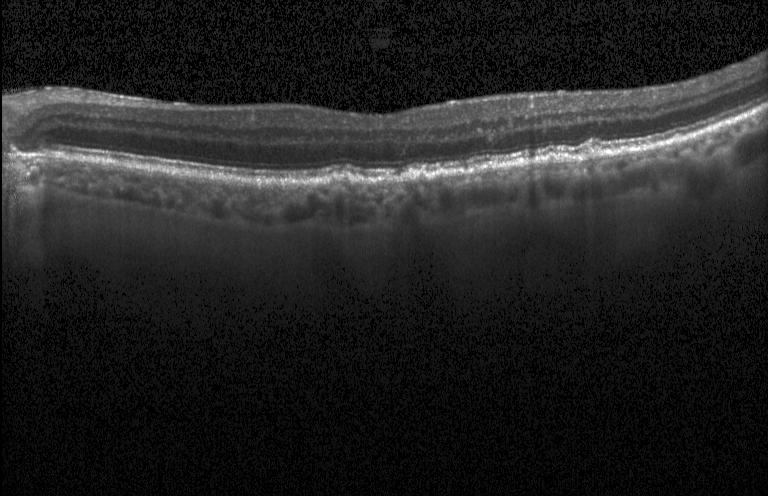 Retinal OCT B-scan, horizontal scan through the fovea, acquired on a Heidelberg Spectralis — DME.